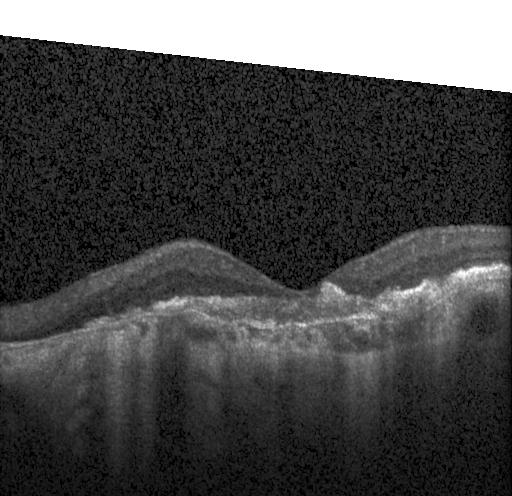

Spectral-domain OCT, macular scan, optical coherence tomography scan
Diagnosis: a choroidal neovascular membrane.